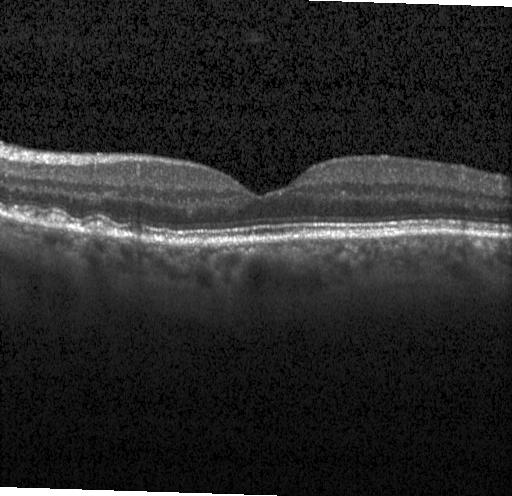
Optical coherence tomography scan — Finding: multiple drusen.